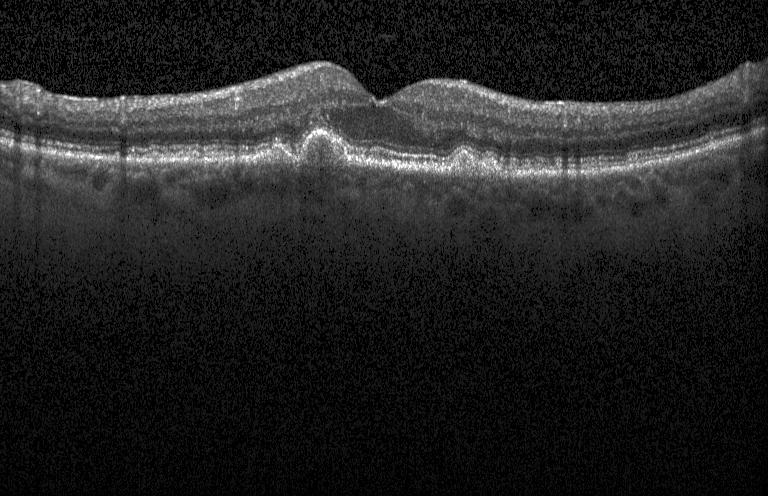
Diagnosis: drusen.